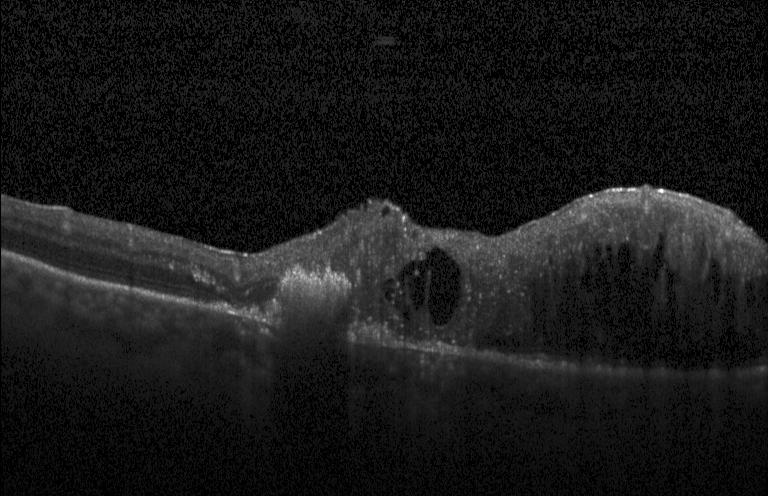
Instrument: Heidelberg Spectralis, SD-OCT, retinal OCT cross-section — The scan shows a choroidal neovascular membrane.